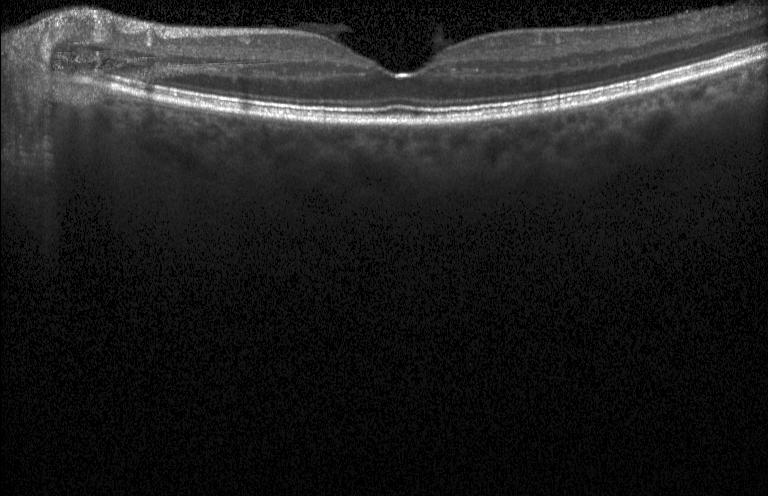 Dx: no choroidal neovascularization, no diabetic macular edema, and no drusen.